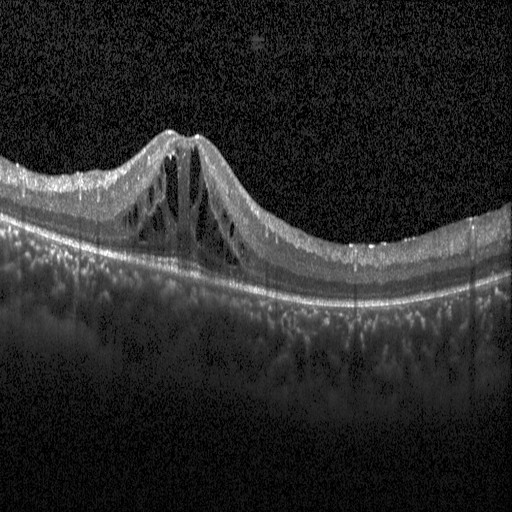
Horizontal scan through the fovea, optical coherence tomography B-scan
Diabetic macular edema.